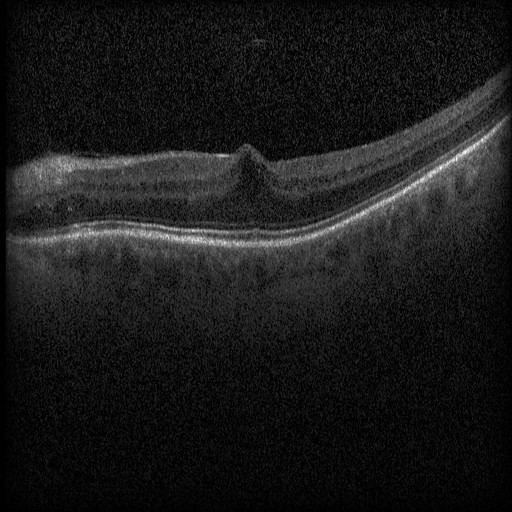

Finding: diabetic macular edema (DME).